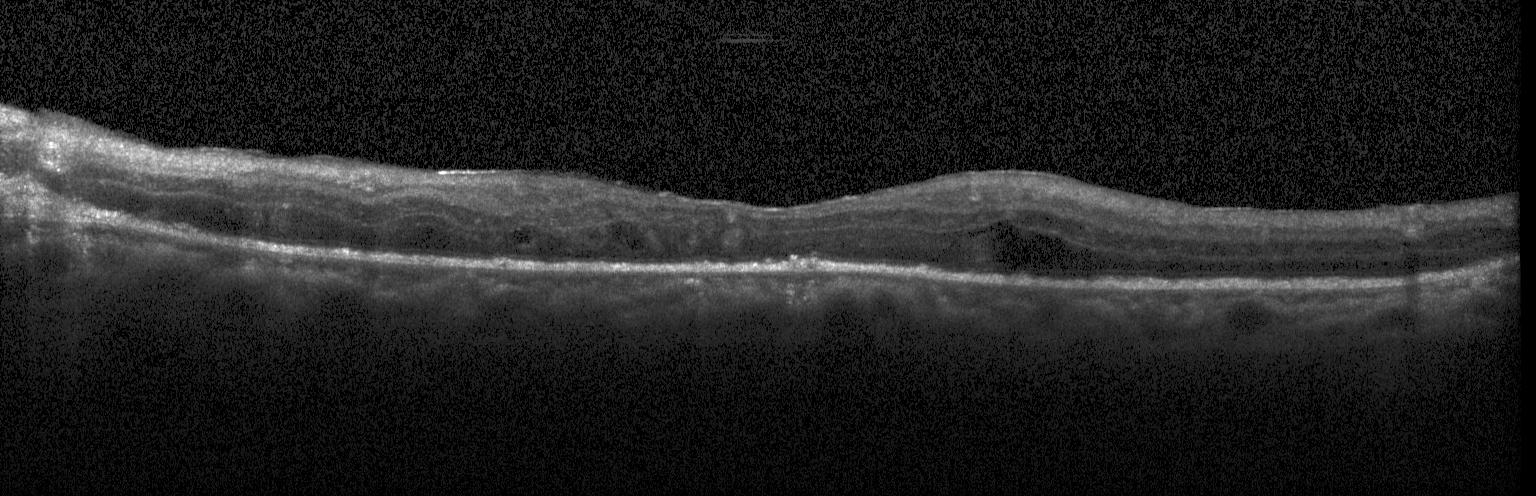

The scan shows DME.